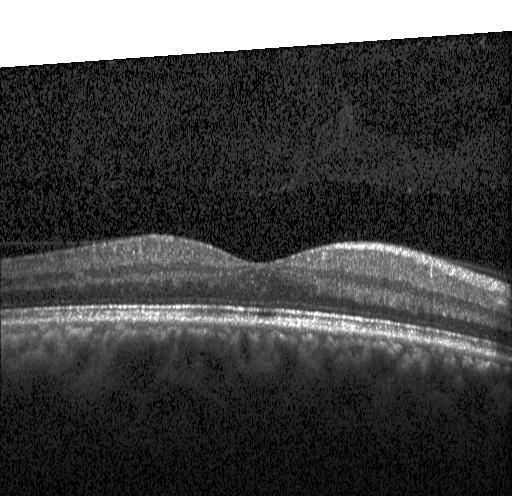 OCT B-scan. Neither choroidal neovascularization, diabetic macular edema, nor drusen.